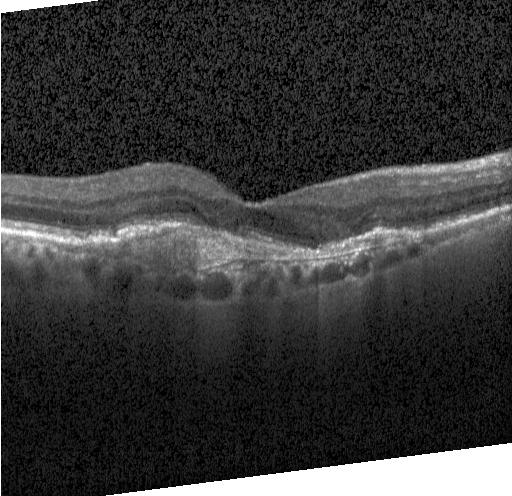
The scan shows choroidal neovascularization (CNV).